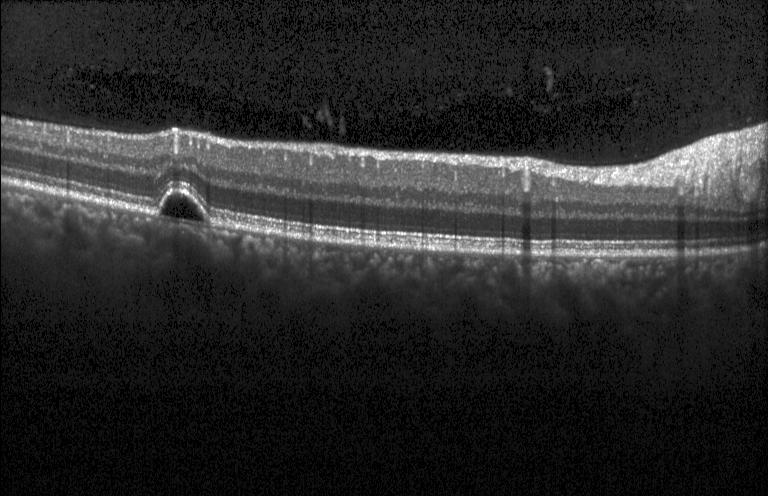 Fovea-centered. Acquired on a Heidelberg Spectralis. Retinal OCT cross-section
Impression: a choroidal neovascular membrane.